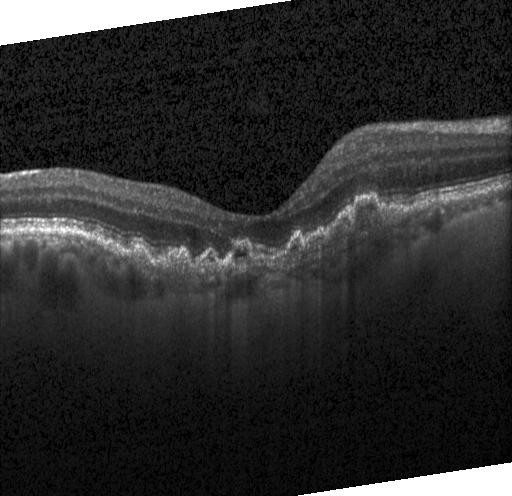 OCT B-scan
Dx: choroidal neovascularization.